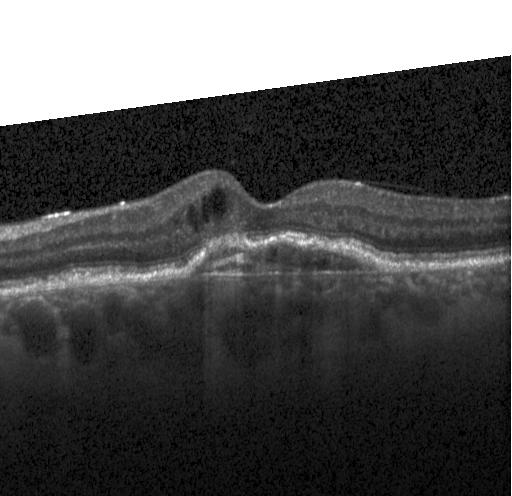 A choroidal neovascular membrane.